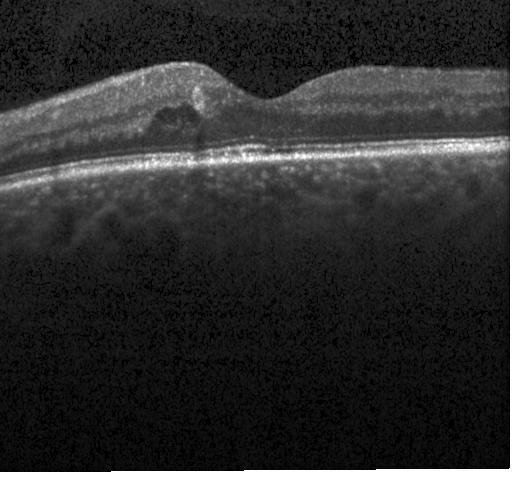

Optical coherence tomography scan. SD-OCT. Heidelberg Spectralis OCT system
Finding: diabetic macular edema (DME).